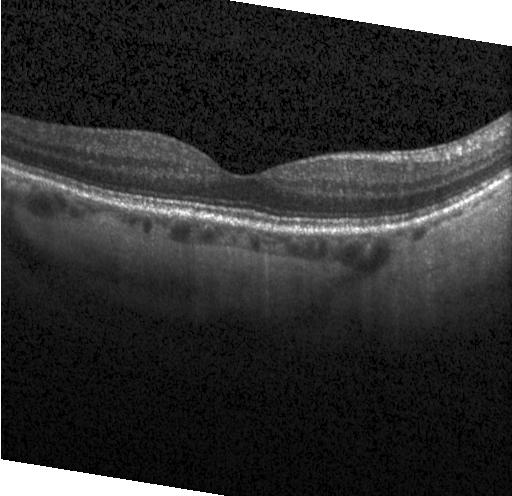

Optical coherence tomography scan. Finding: neither choroidal neovascularization, diabetic macular edema, nor drusen.